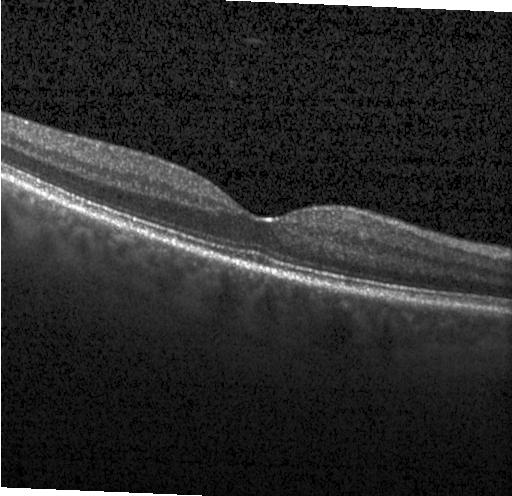 Centered on the fovea; spectral-domain OCT; optical coherence tomography B-scan; acquired on a Heidelberg Spectralis.
Assessment: no CNV, no DME, and no drusen.